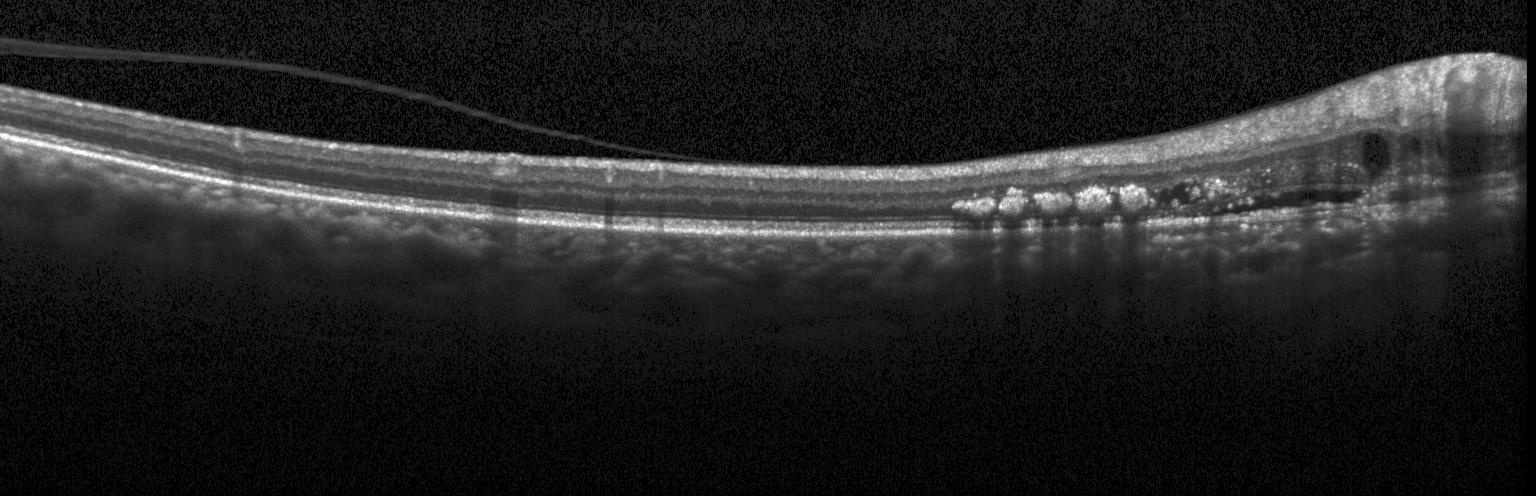 Through the macula. SD-OCT. OCT B-scan. Instrument: Heidelberg Spectralis — Choroidal neovascularization (CNV).